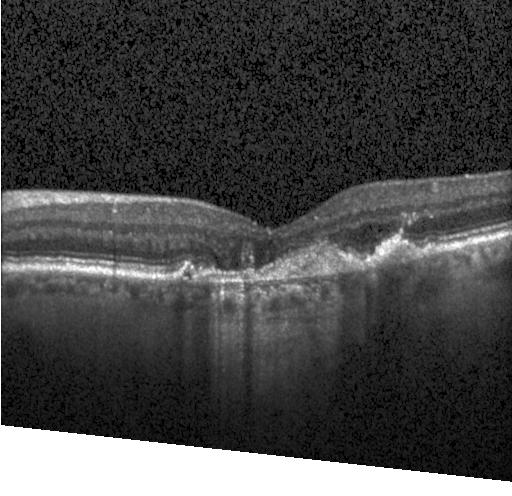 Instrument: Heidelberg Spectralis, optical coherence tomography scan. Finding: CNV.